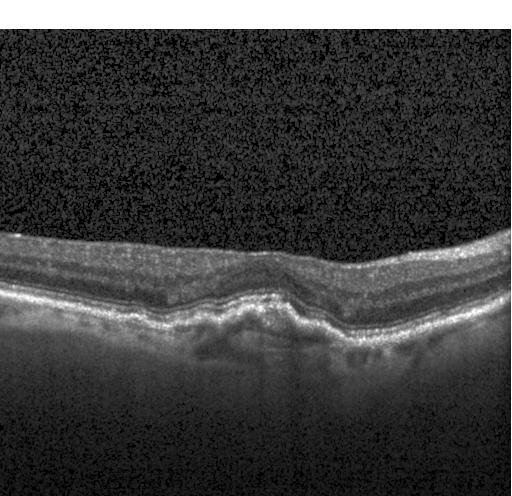

Spectral-domain OCT; centered on the fovea; instrument: Heidelberg Spectralis; OCT B-scan
A choroidal neovascular membrane.